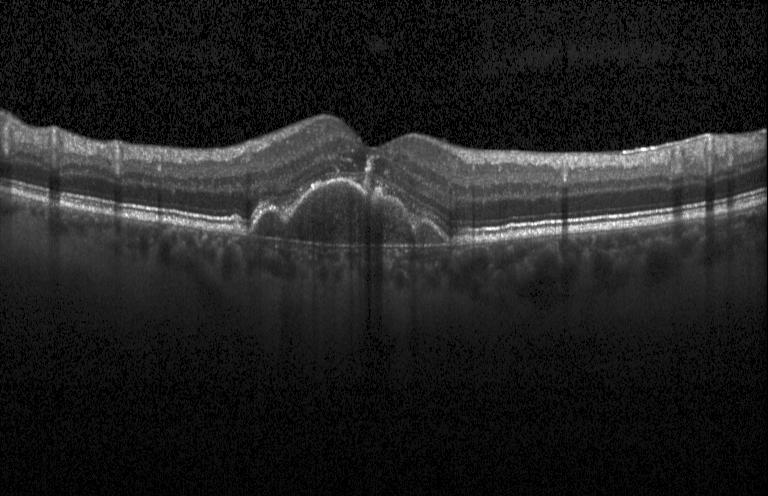 Retinal OCT B-scan.
Diagnosis: CNV.